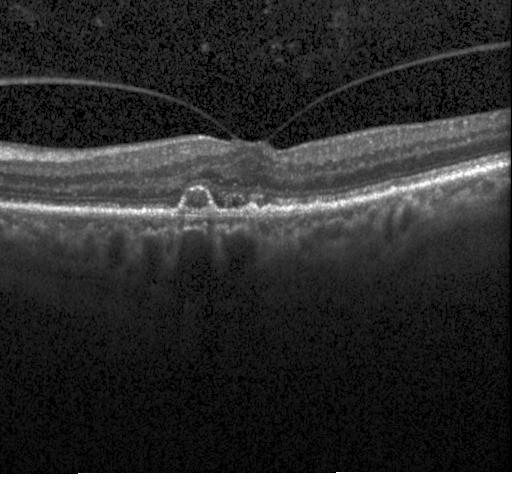 Instrument: Heidelberg Spectralis, spectral-domain optical coherence tomography, retinal OCT B-scan, through the macula — Impression: a choroidal neovascular membrane.